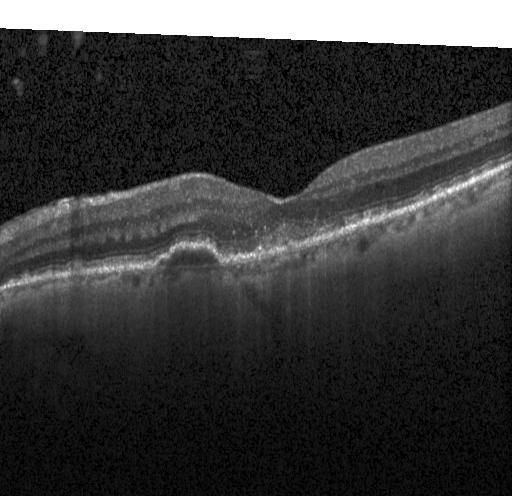
SD-OCT · macular scan · OCT B-scan.
This B-scan demonstrates CNV.